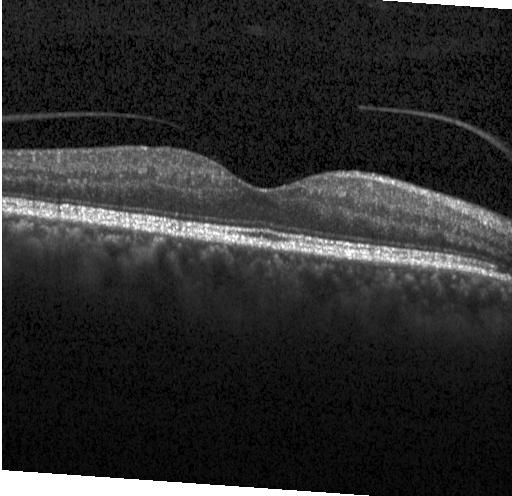 Centered on the fovea, SD-OCT, Heidelberg Spectralis, retinal OCT B-scan.
OCT finding: no evidence of choroidal neovascularization, diabetic macular edema, or drusen.